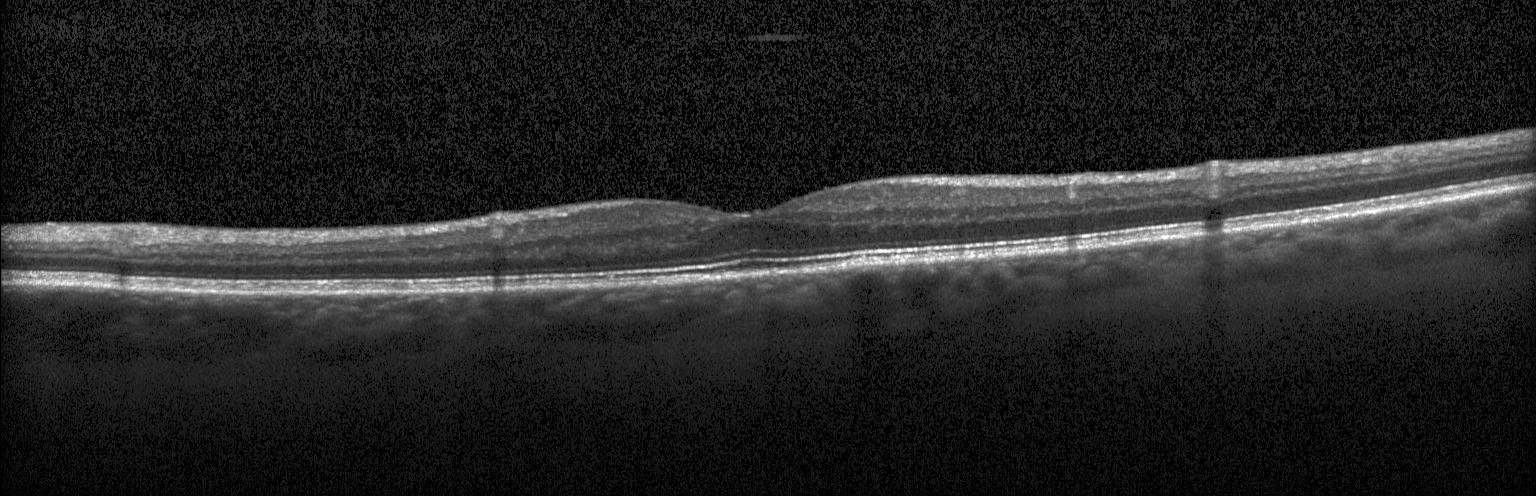
Through the macula · optical coherence tomography scan · spectral-domain optical coherence tomography.
Diagnosis: no choroidal neovascularization, no diabetic macular edema, and no drusen.